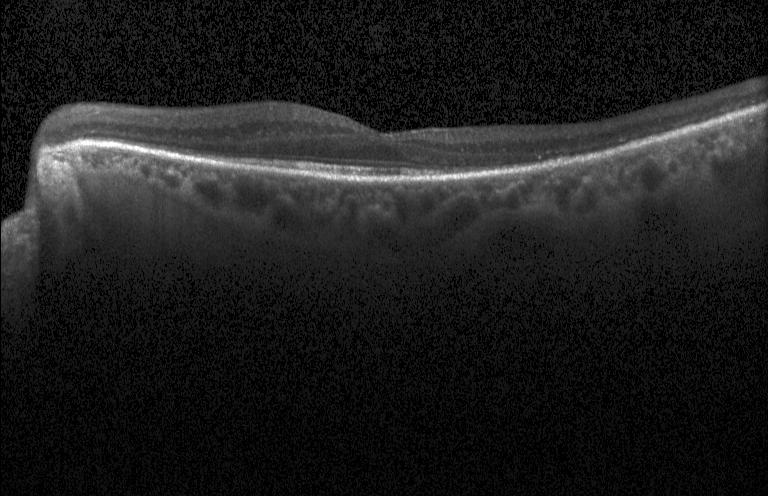 Spectral-domain OCT B-scan: no evidence of CNV, DME, or drusen.